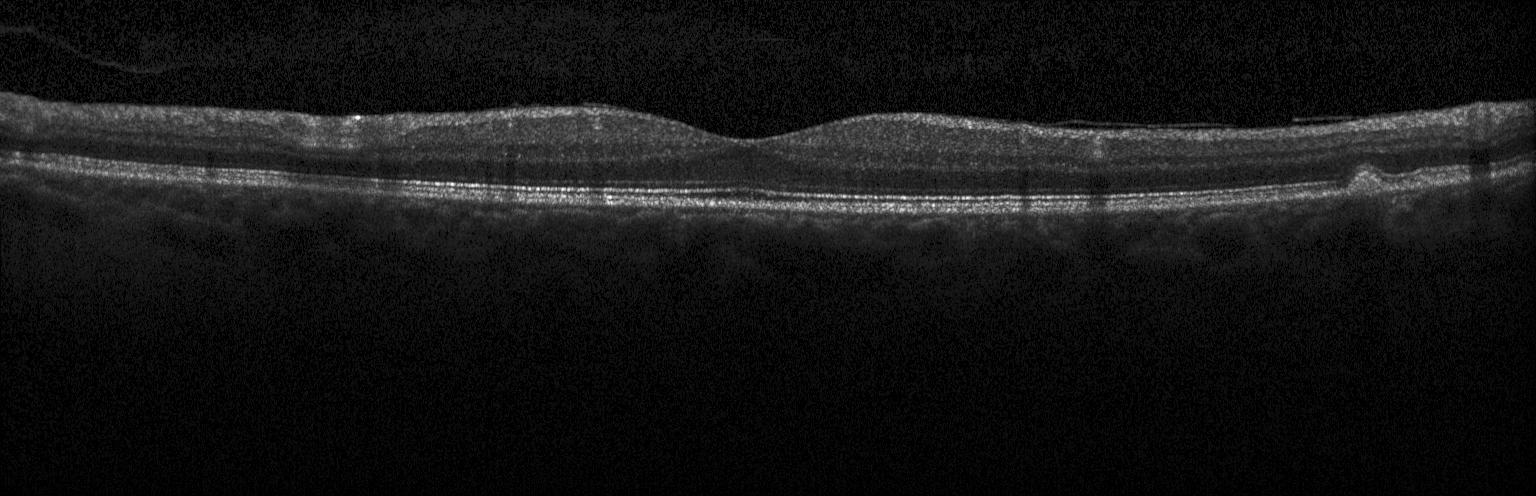
Impression: multiple drusen.